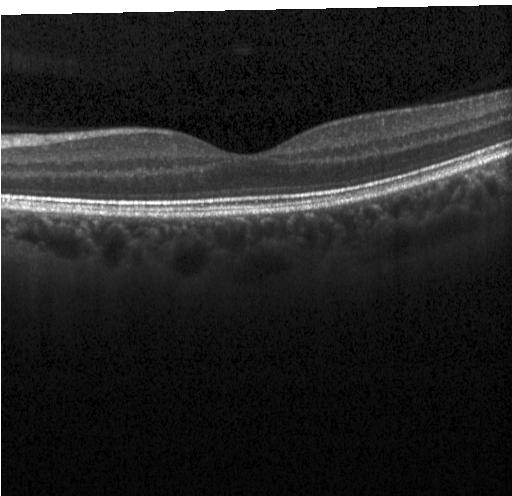

Optical coherence tomography B-scan; spectral-domain OCT; through the macula — Dx: no CNV, DME, or drusen.